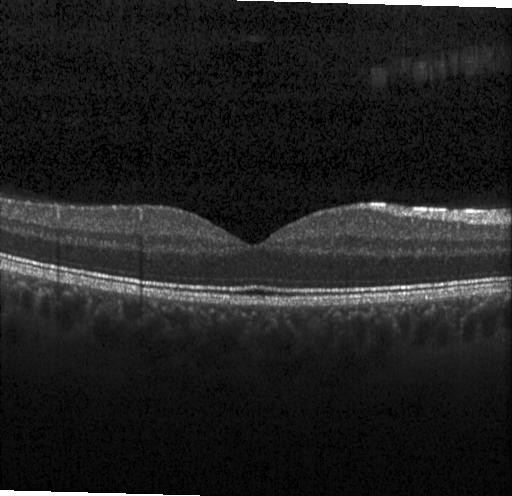

Diagnosis: no evidence of choroidal neovascularization, diabetic macular edema, or drusen.